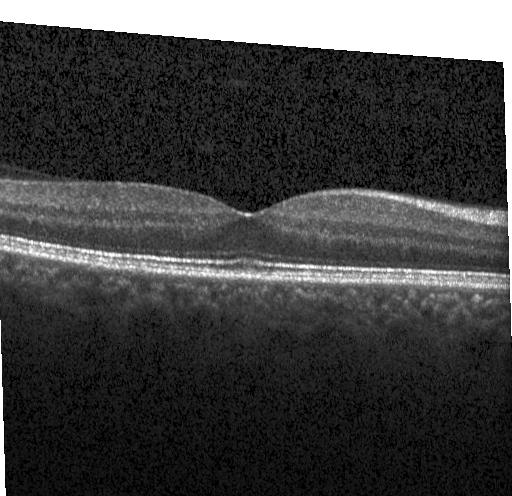

Through the macula · spectral-domain optical coherence tomography · instrument: Heidelberg Spectralis · optical coherence tomography scan
OCT finding: no CNV, DME, or drusen.